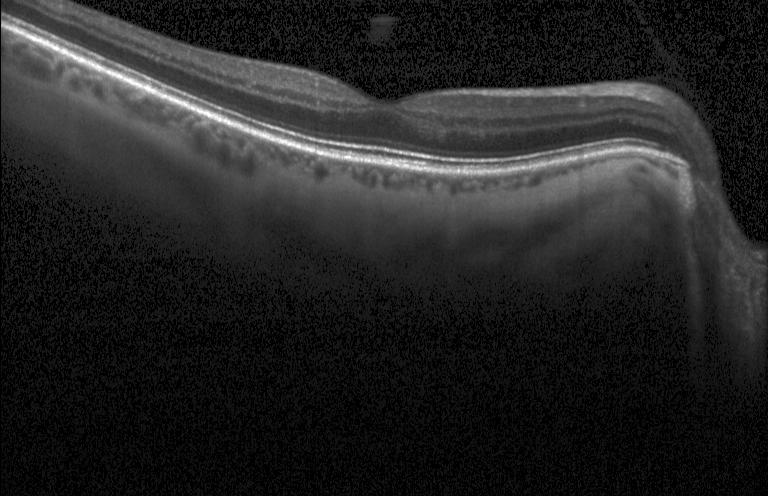

Macular scan; spectral-domain OCT; acquired on a Heidelberg Spectralis; retinal OCT cross-section — Assessment: no CNV, DME, or drusen.